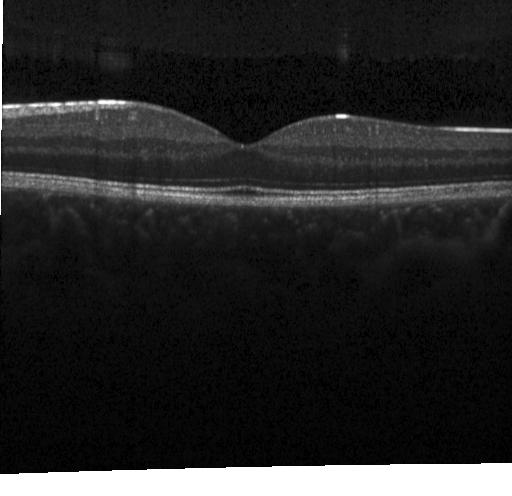
Spectral-domain optical coherence tomography. Optical coherence tomography B-scan — Diagnosis: no choroidal neovascularization, no diabetic macular edema, and no drusen.